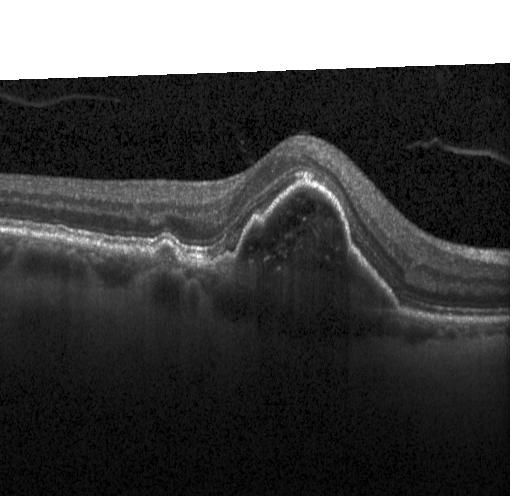

Spectral-domain OCT, acquired on a Heidelberg Spectralis, horizontal scan through the fovea, OCT line scan
This B-scan demonstrates a choroidal neovascular membrane.